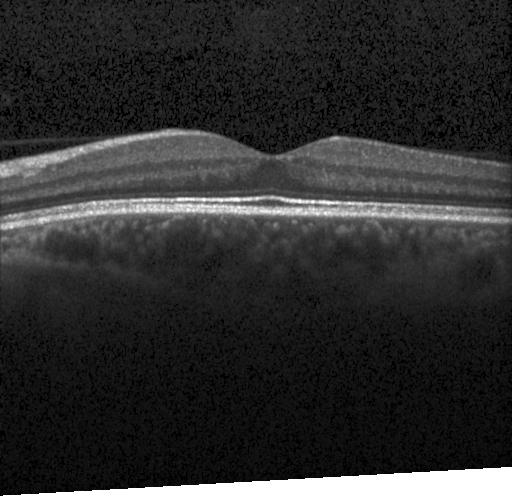
Heidelberg Spectralis, optical coherence tomography B-scan.
Neither CNV, DME, nor drusen.